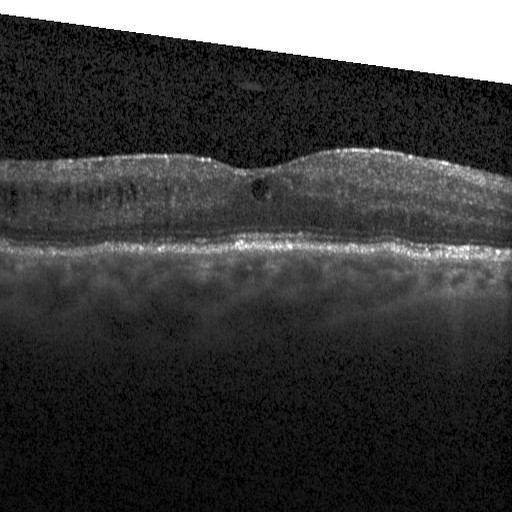

OCT finding: diabetic macular edema (DME).